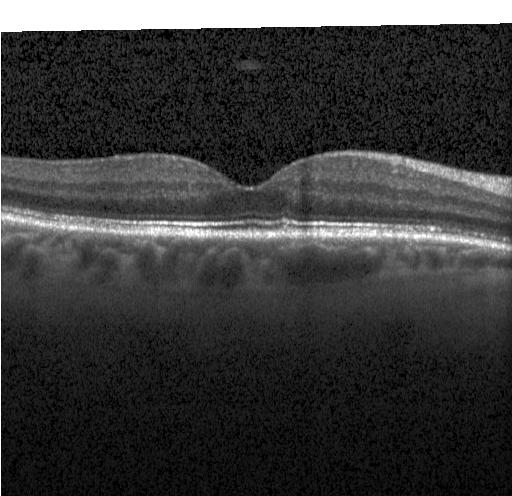
Centered on the fovea. Optical coherence tomography scan.
Finding: no evidence of choroidal neovascularization, diabetic macular edema, or drusen.